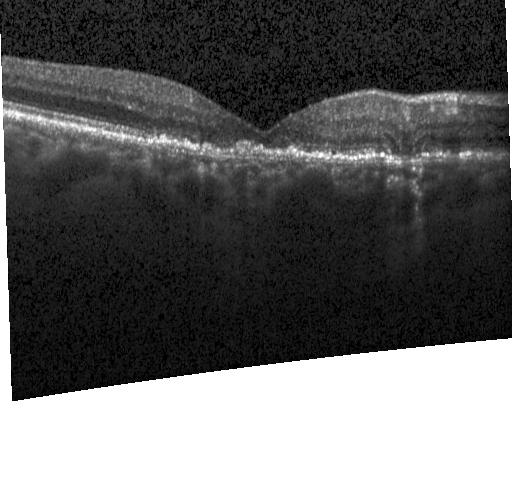
Macular OCT demonstrating a choroidal neovascular membrane.